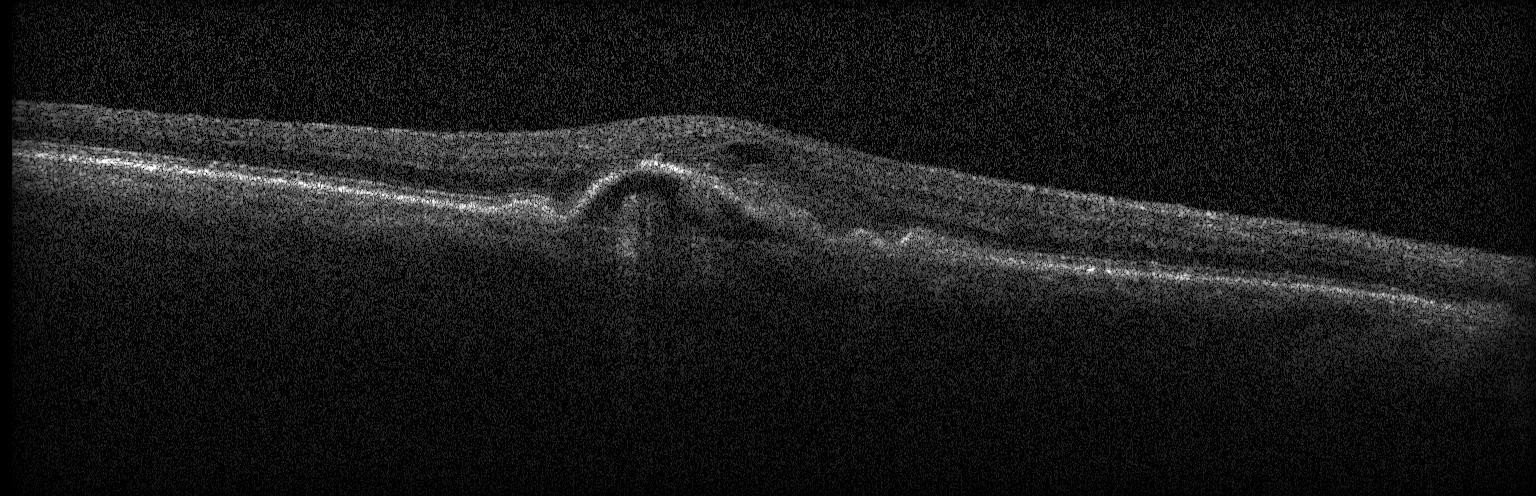
OCT line scan — Finding: a choroidal neovascular membrane.